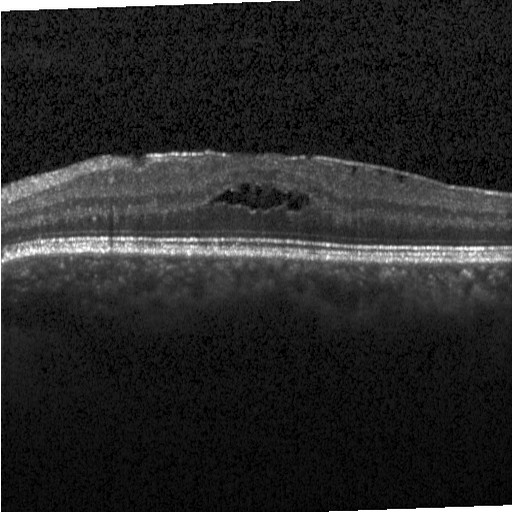
Retinal OCT B-scan; Heidelberg Spectralis OCT system; macular scan; spectral-domain optical coherence tomography — Diagnosis: DME.